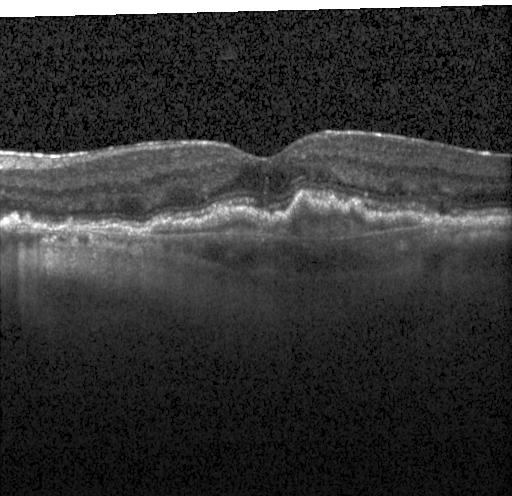
Heidelberg Spectralis OCT system, optical coherence tomography B-scan, spectral-domain OCT, centered on the fovea
Diagnosis: CNV.